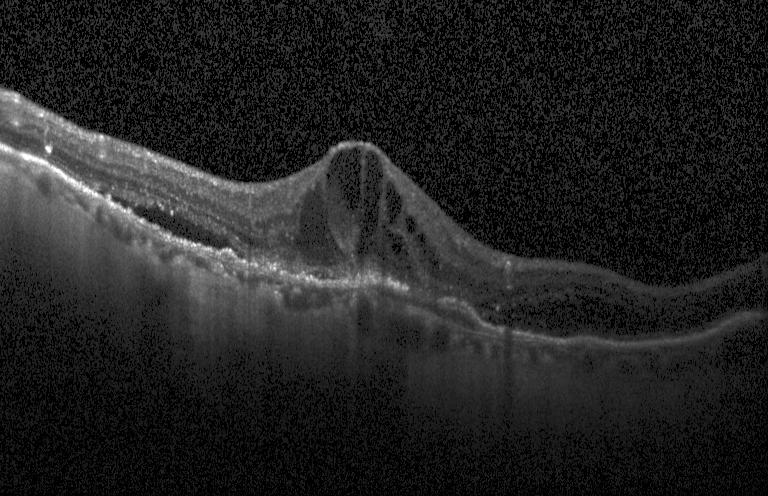

Optical coherence tomography B-scan, acquired on a Heidelberg Spectralis
Diagnosis: CNV.